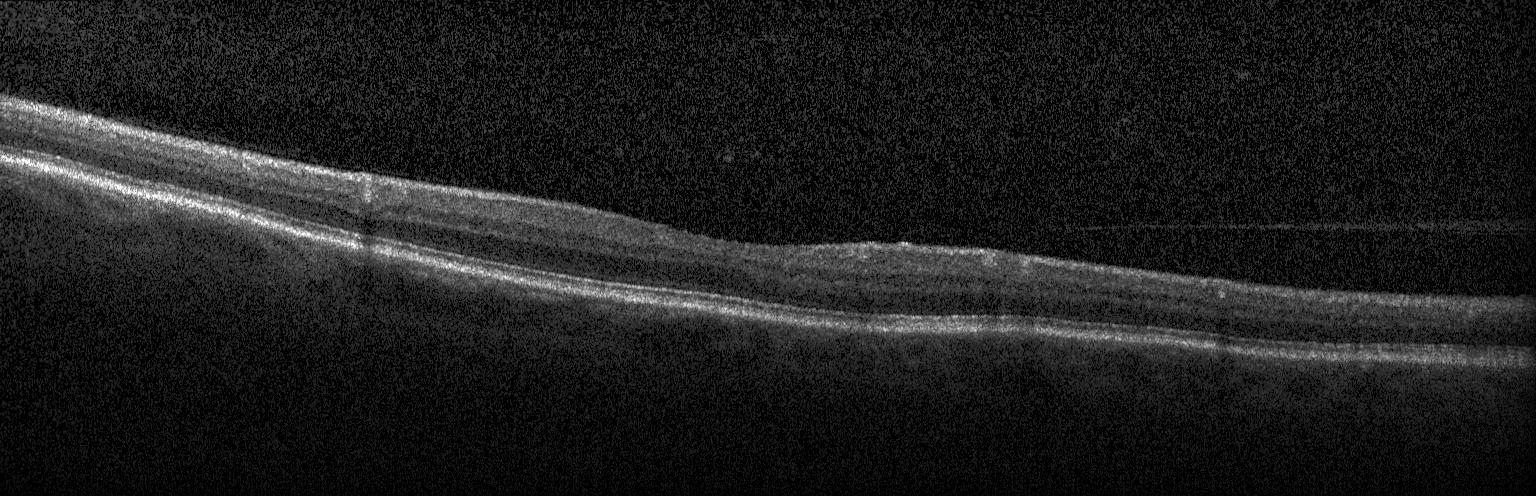
Macular OCT demonstrating neither CNV, DME, nor drusen.